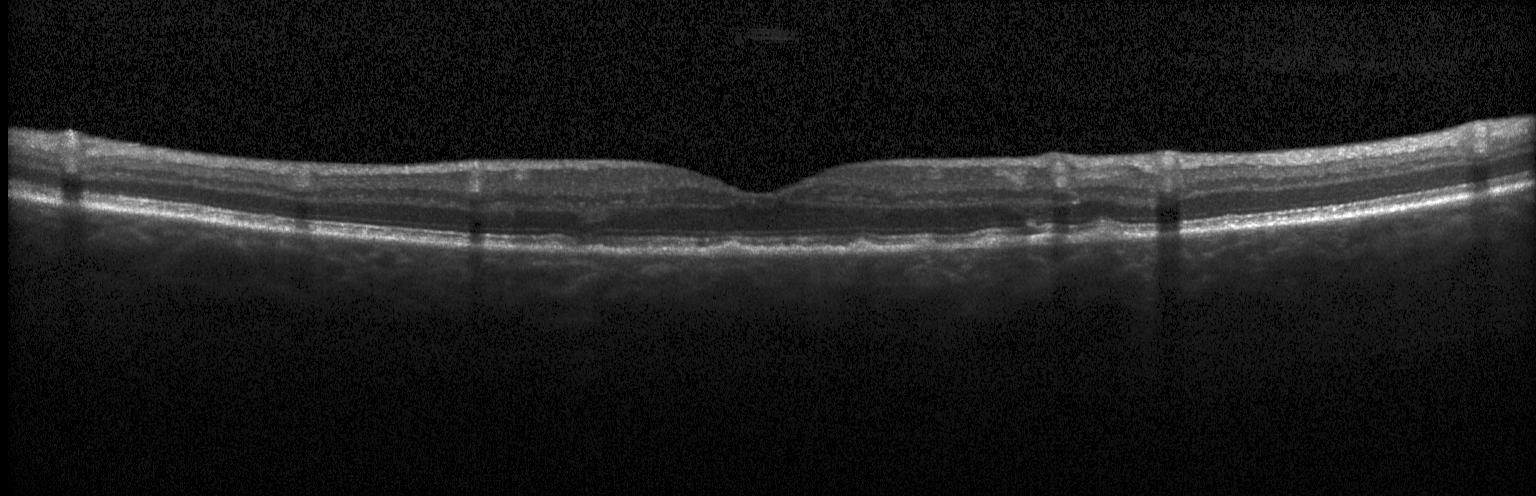

OCT line scan — Dx: drusen.